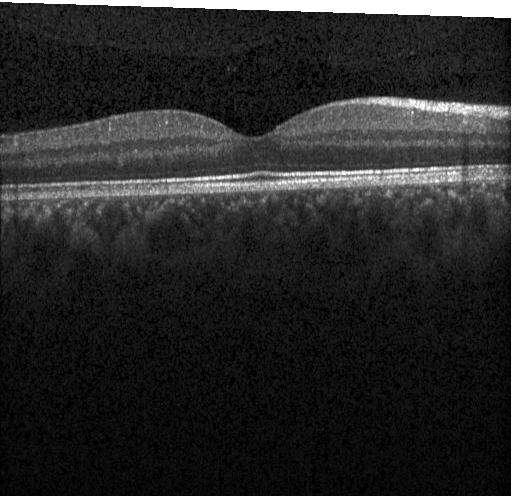
SD-OCT; Heidelberg Spectralis; centered on the fovea; optical coherence tomography B-scan.
Impression: no choroidal neovascularization, no diabetic macular edema, and no drusen.